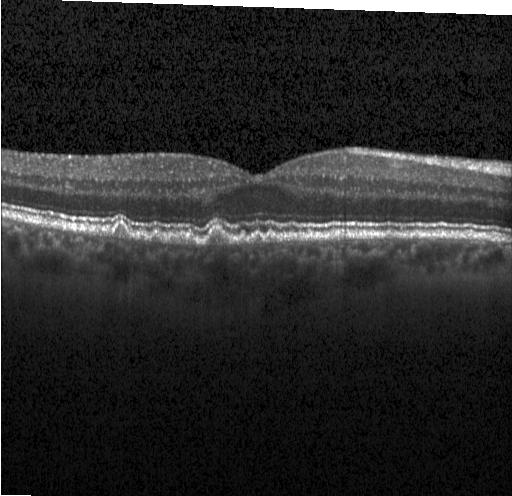 Optical coherence tomography B-scan · spectral-domain optical coherence tomography
Sub-RPE drusenoid deposits.